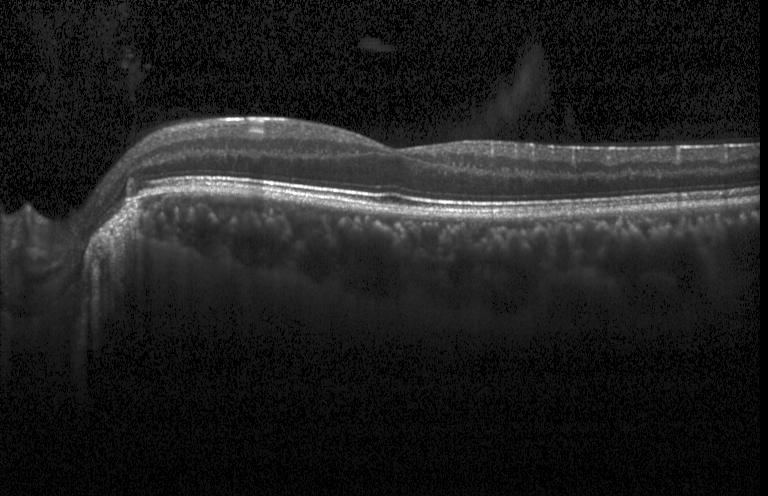

Finding: no evidence of choroidal neovascularization, diabetic macular edema, or drusen.